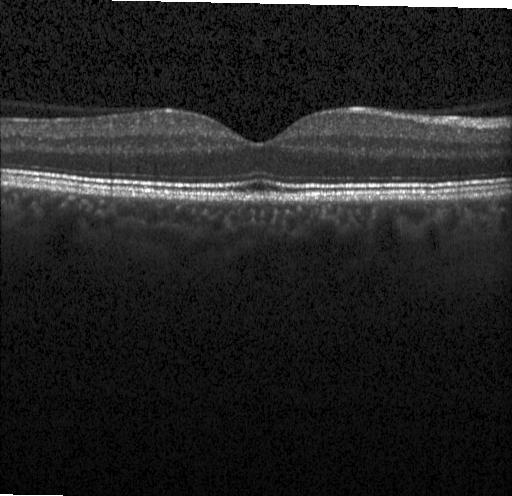 Macular OCT: no evidence of CNV, DME, or drusen.